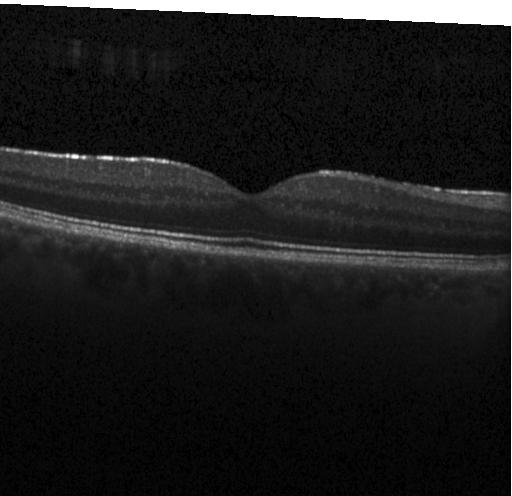
Horizontal scan through the fovea, SD-OCT, retinal OCT cross-section. Assessment: neither choroidal neovascularization, diabetic macular edema, nor drusen.